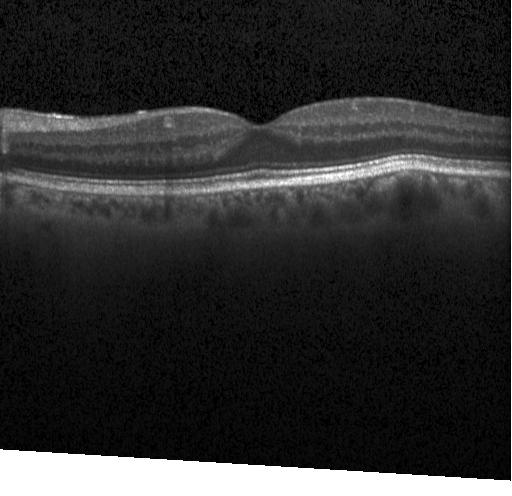
OCT line scan; Heidelberg Spectralis OCT system.
OCT finding: neither CNV, DME, nor drusen.